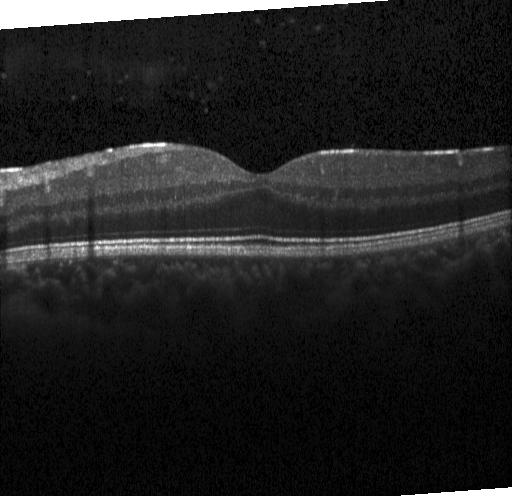
Macular OCT: neither choroidal neovascularization, diabetic macular edema, nor drusen.